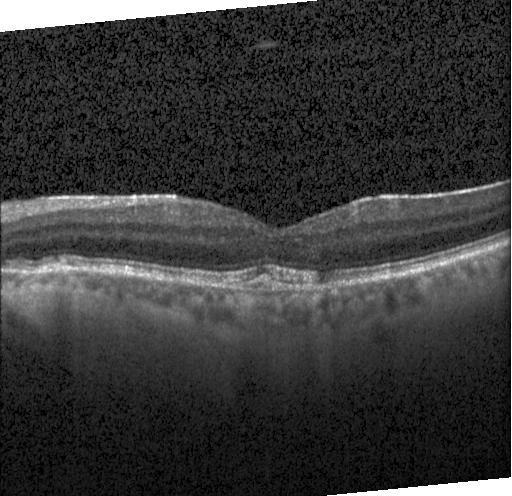 Optical coherence tomography B-scan. OCT finding: CNV.